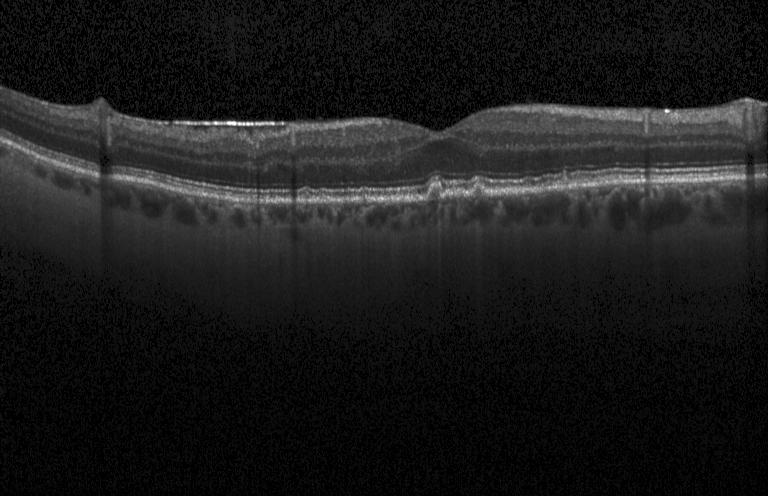

OCT finding: drusen.